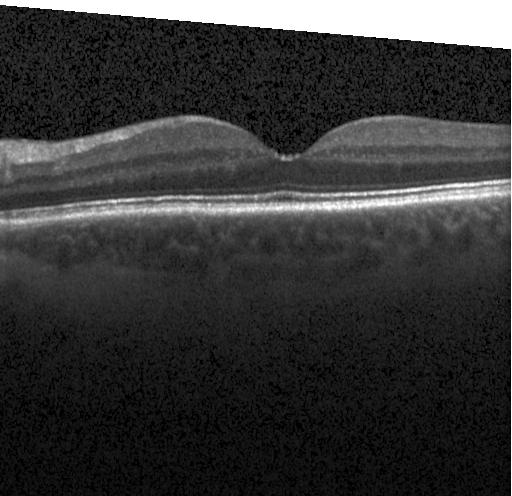

Horizontal scan through the fovea · acquired on a Heidelberg Spectralis · retinal OCT B-scan — This B-scan demonstrates no evidence of choroidal neovascularization, diabetic macular edema, or drusen.